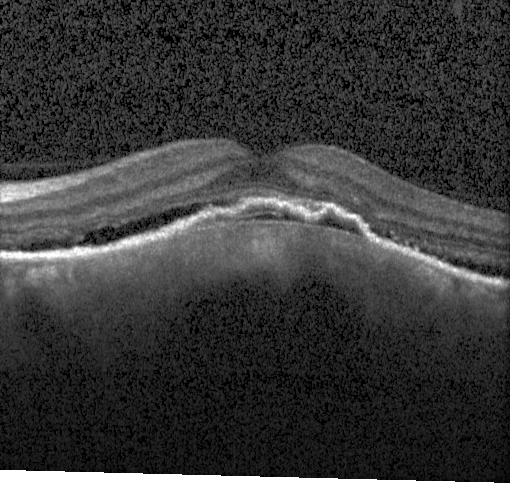 Retinal OCT cross-section — Impression: choroidal neovascularization.